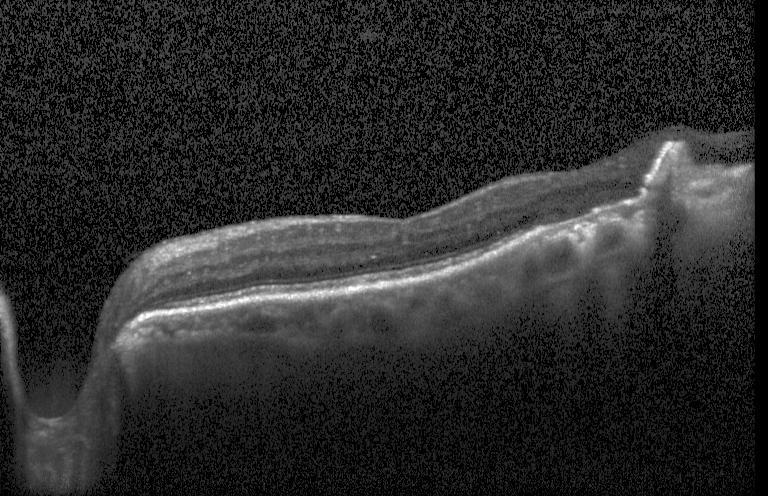 Optical coherence tomography scan. Heidelberg Spectralis. SD-OCT — Diagnosis: choroidal neovascularization (CNV).